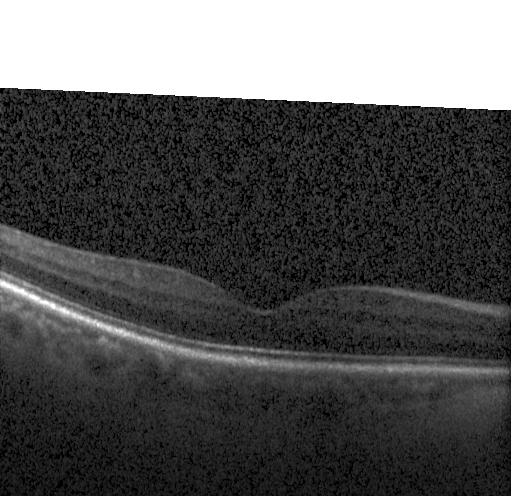
SD-OCT · optical coherence tomography B-scan · acquired on a Heidelberg Spectralis. Diagnosis: no choroidal neovascularization, no diabetic macular edema, and no drusen.